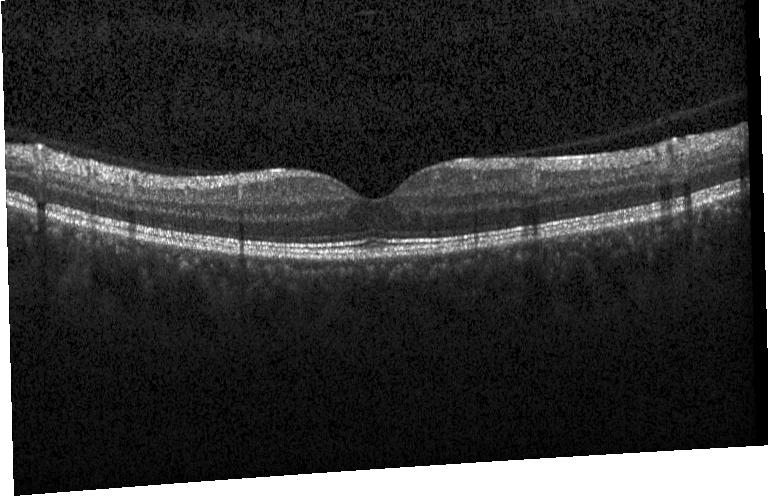

OCT B-scan · macular scan · acquired on a Heidelberg Spectralis
Neither choroidal neovascularization, diabetic macular edema, nor drusen.